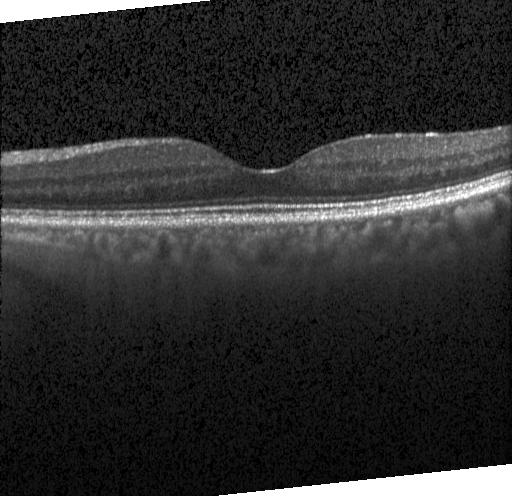

Instrument: Heidelberg Spectralis, horizontal scan through the fovea, optical coherence tomography B-scan, spectral-domain OCT
The scan shows no choroidal neovascularization, diabetic macular edema, or drusen.